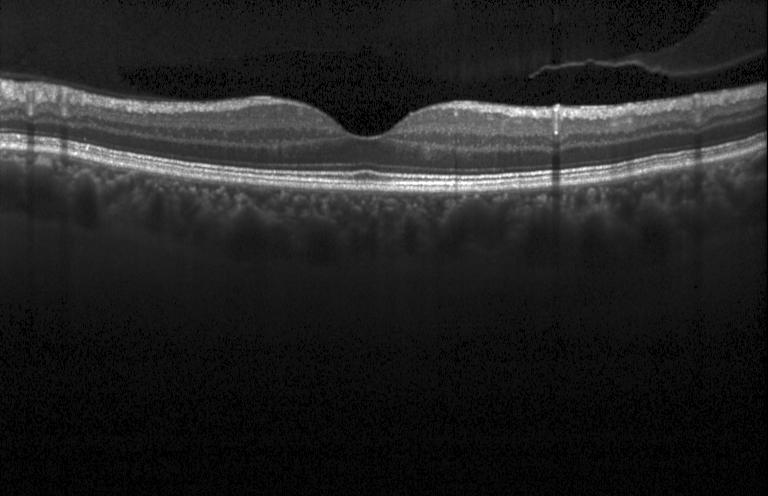

Diagnosis: neither CNV, DME, nor drusen.